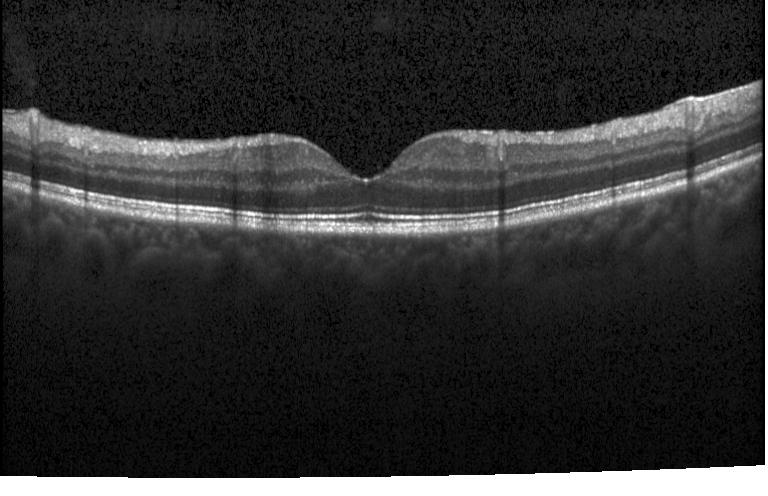
Retinal OCT cross-section showing no CNV, no DME, and no drusen.